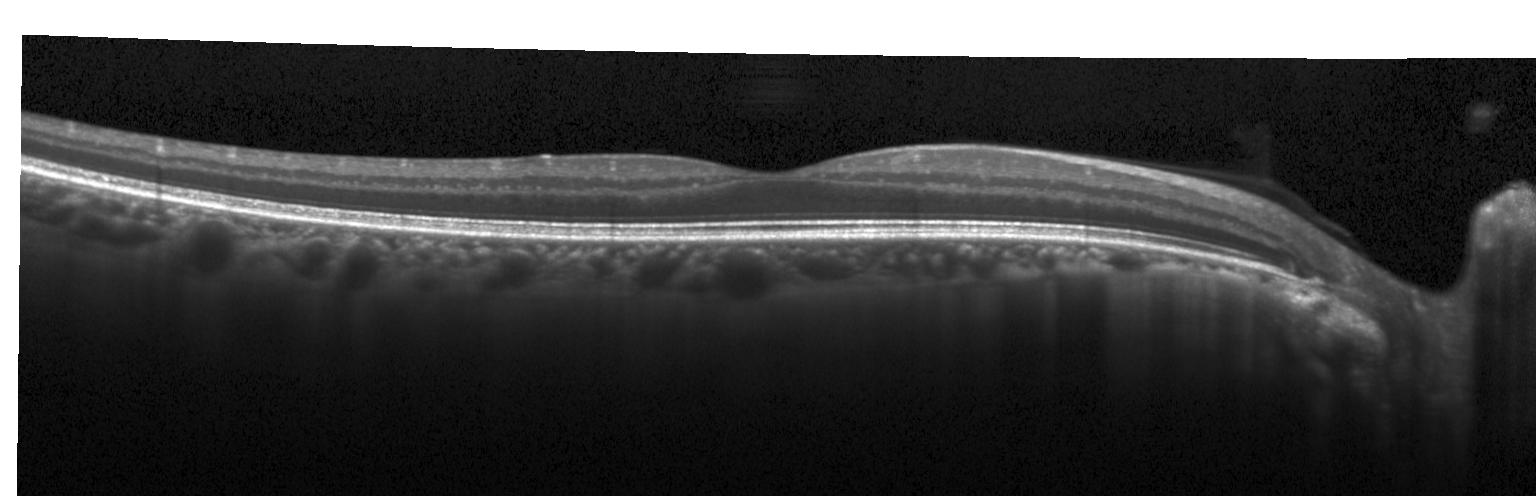 Finding: no evidence of choroidal neovascularization, diabetic macular edema, or drusen.